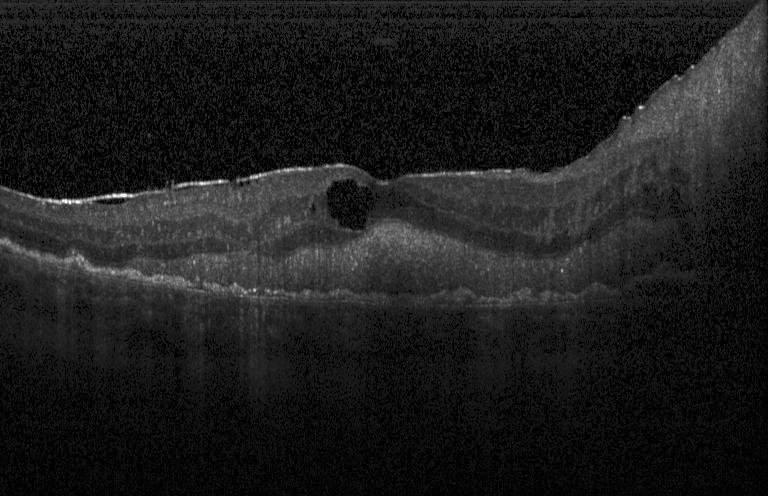

Macular scan. Heidelberg Spectralis. SD-OCT. Retinal OCT B-scan. Impression: a choroidal neovascular membrane.